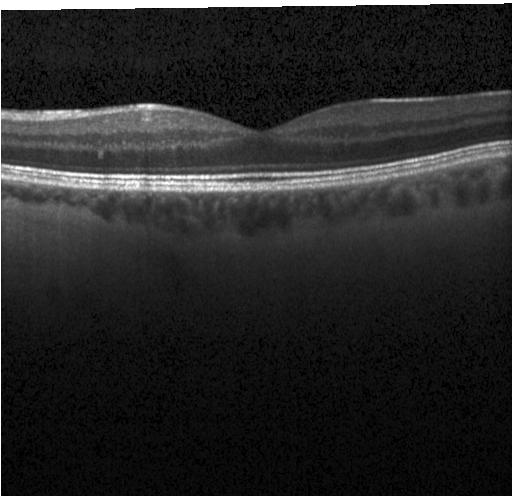

SD-OCT; OCT line scan; macular scan.
This B-scan demonstrates no evidence of choroidal neovascularization, diabetic macular edema, or drusen.